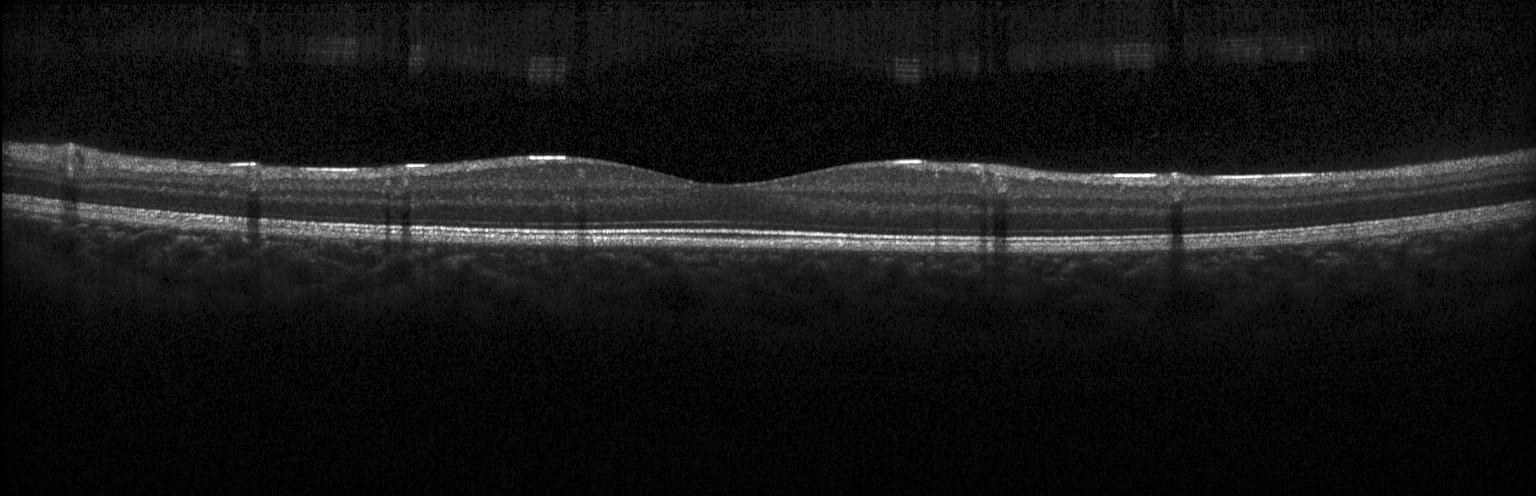
Diagnosis: no choroidal neovascularization, diabetic macular edema, or drusen.